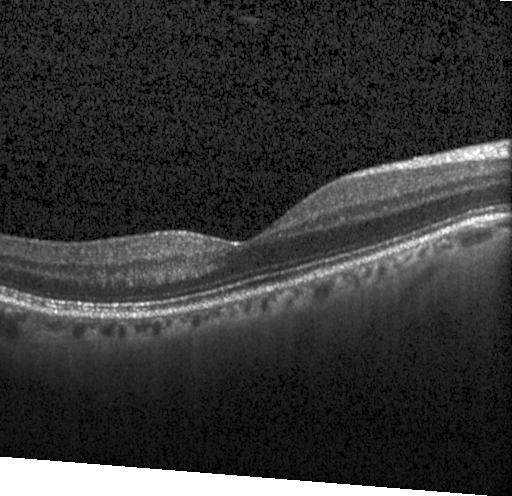
Centered on the fovea; Heidelberg Spectralis; OCT line scan. This B-scan demonstrates neither choroidal neovascularization, diabetic macular edema, nor drusen.